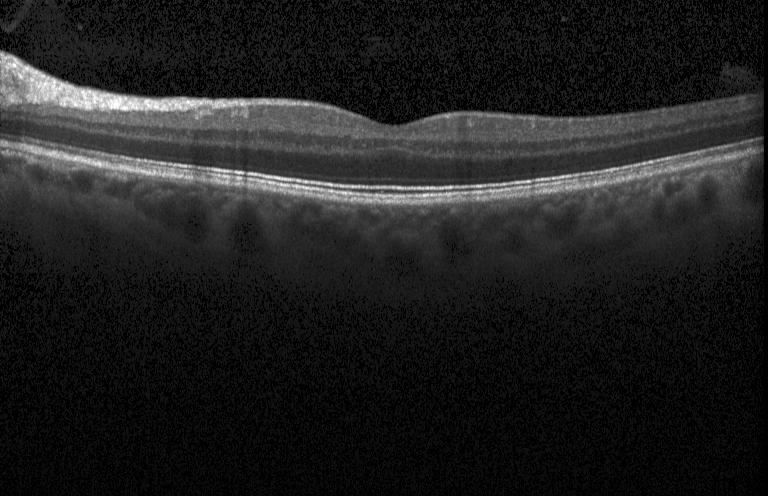 Retinal OCT cross-section. Horizontal scan through the fovea.
The scan shows no choroidal neovascularization, diabetic macular edema, or drusen.